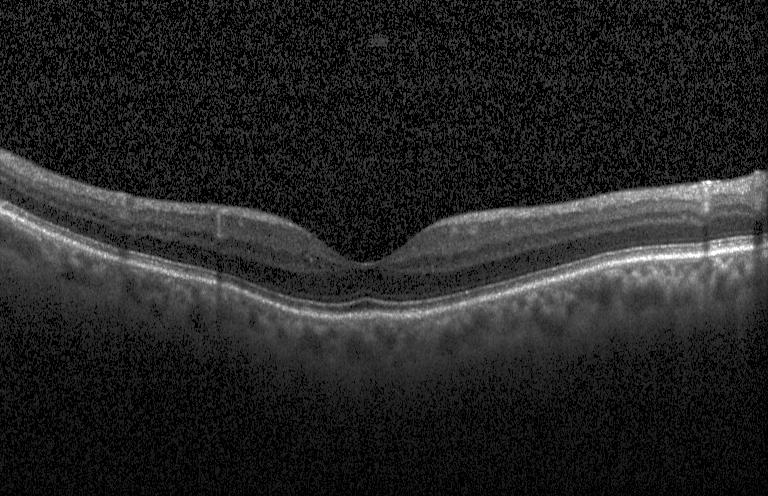 Finding: no CNV, DME, or drusen.